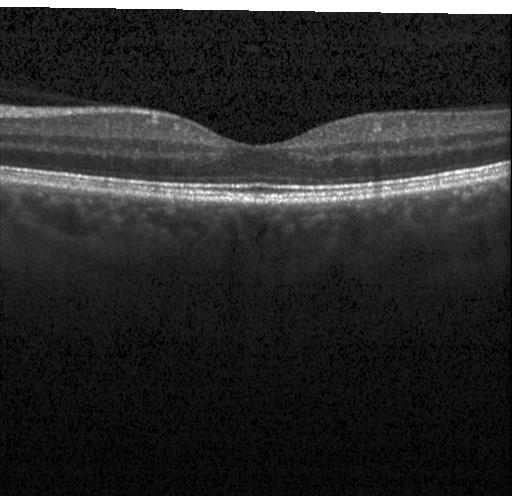
Optical coherence tomography B-scan.
Macular OCT: neither choroidal neovascularization, diabetic macular edema, nor drusen.